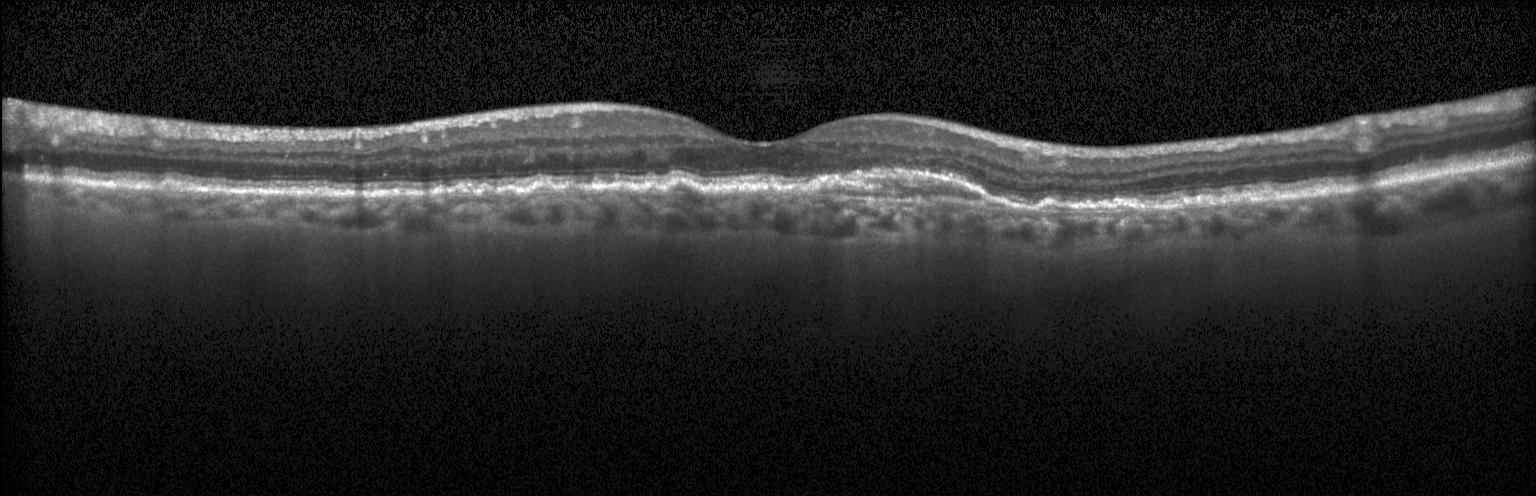
Retinal OCT B-scan; macular scan. Choroidal neovascularization.